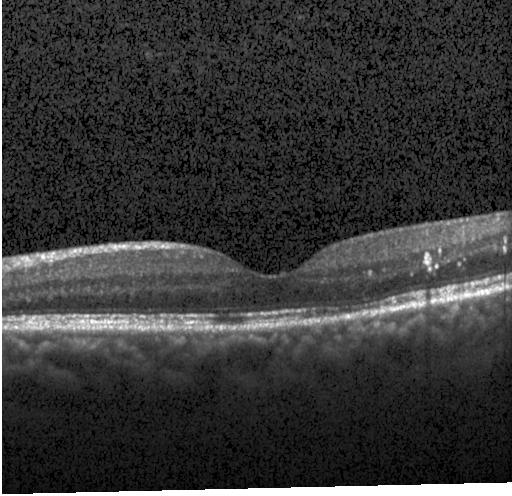

Assessment: diabetic macular edema.